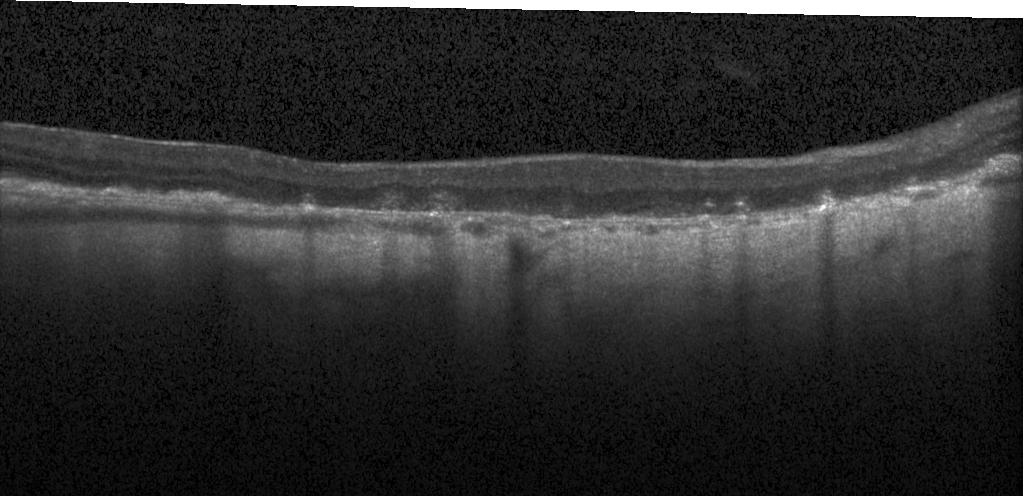
No choroidal neovascularization, no diabetic macular edema, and no drusen.